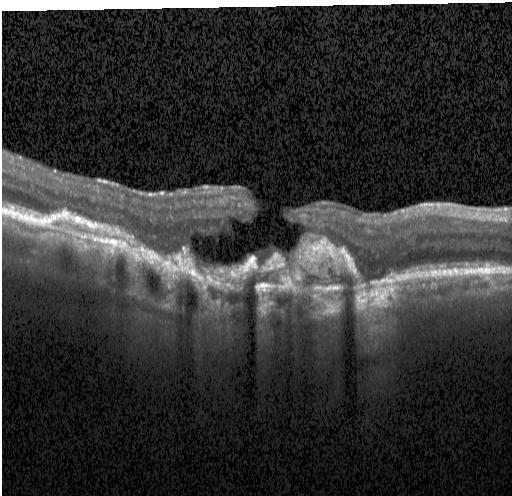
Spectral-domain OCT B-scan: a choroidal neovascular membrane.